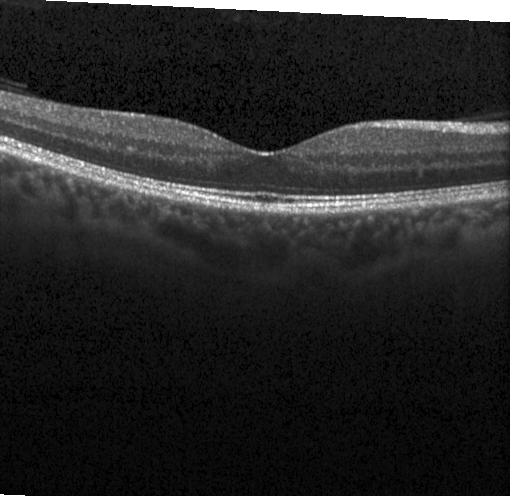
Horizontal scan through the fovea · OCT B-scan · instrument: Heidelberg Spectralis · spectral-domain OCT.
Diagnosis: no evidence of choroidal neovascularization, diabetic macular edema, or drusen.